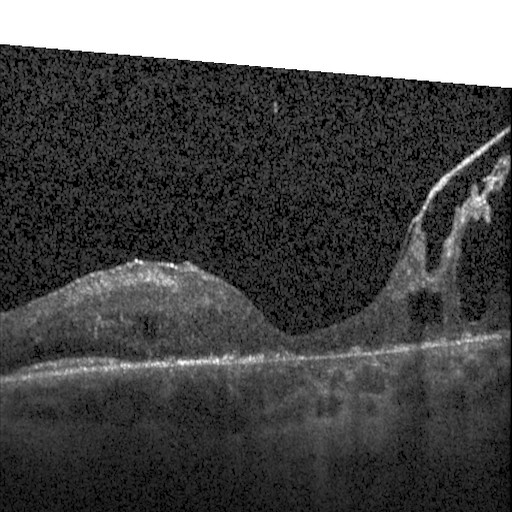 Heidelberg Spectralis. OCT B-scan. Centered on the fovea. SD-OCT.
This B-scan demonstrates diabetic macular edema (DME).